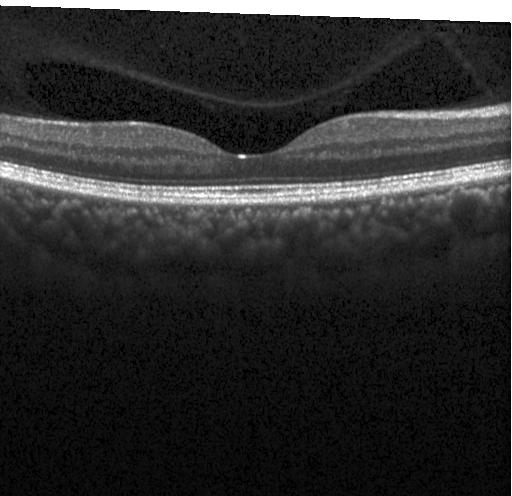
Optical coherence tomography scan. The scan shows no evidence of CNV, DME, or drusen.